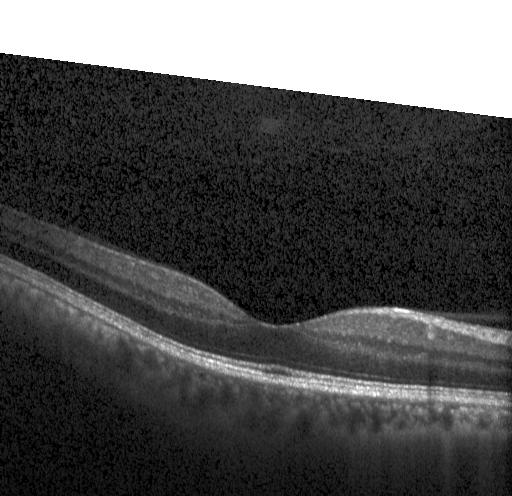 OCT B-scan showing no CNV, no DME, and no drusen.